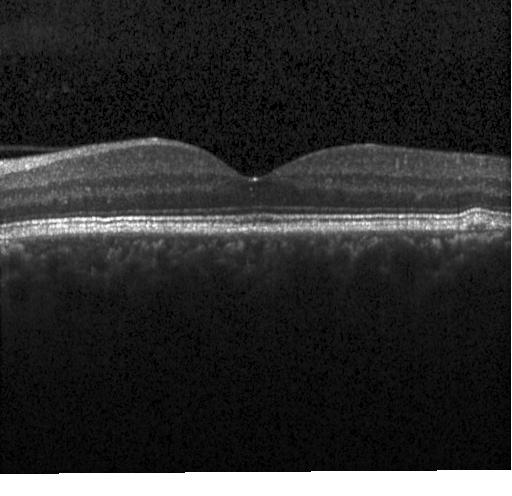
OCT line scan — OCT finding: neither choroidal neovascularization, diabetic macular edema, nor drusen.